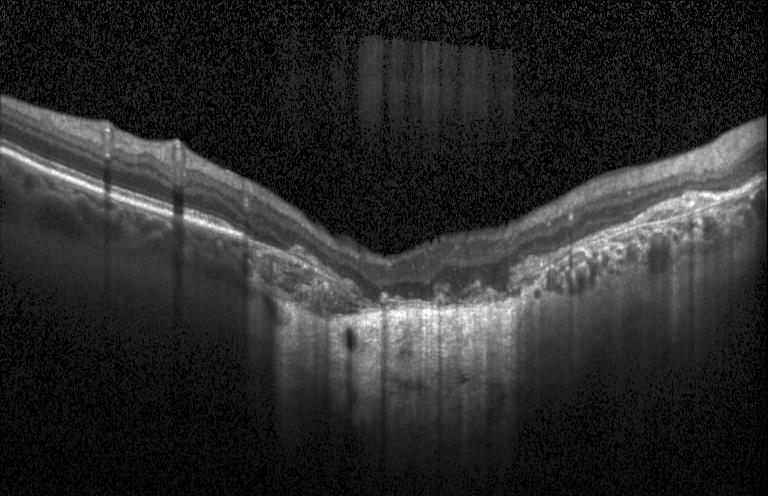 Macular OCT demonstrating a choroidal neovascular membrane.